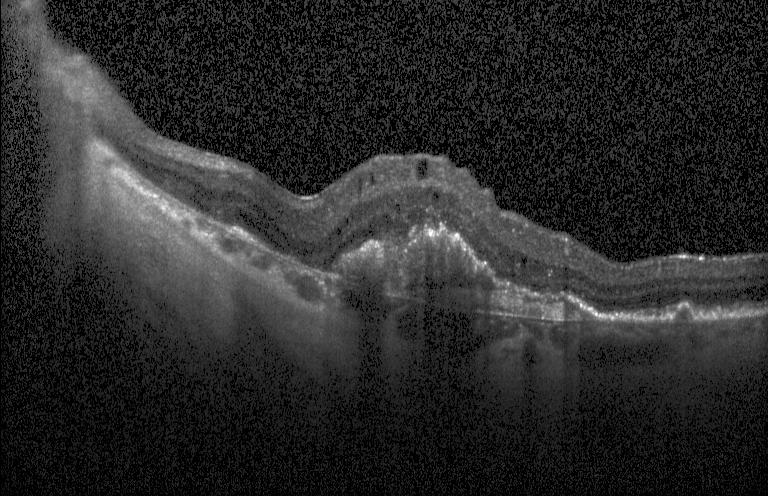
Spectral-domain OCT, retinal OCT B-scan. Assessment: a choroidal neovascular membrane.